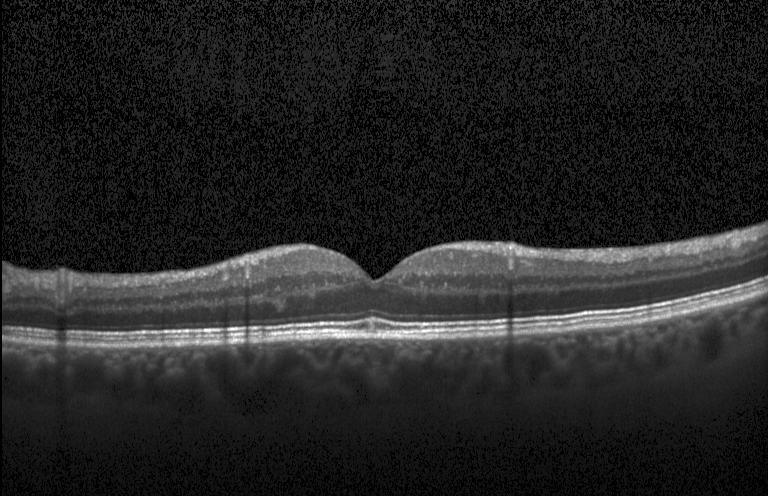 OCT B-scan · Heidelberg Spectralis — OCT finding: no choroidal neovascularization, no diabetic macular edema, and no drusen.